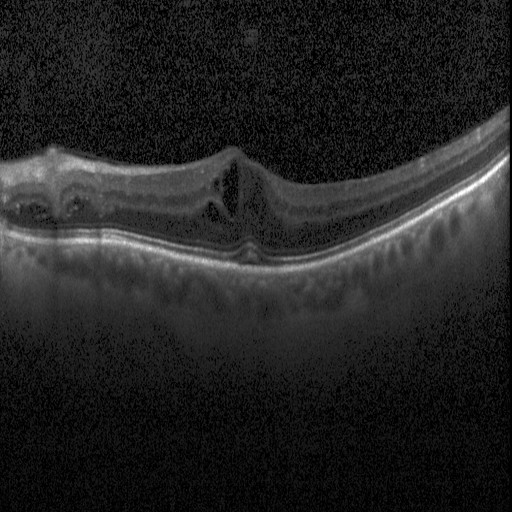 OCT line scan
OCT finding: diabetic macular edema.